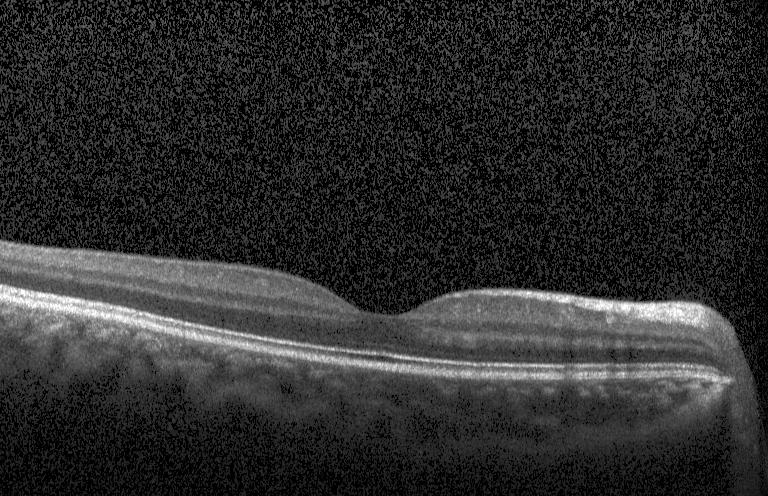

Acquired on a Heidelberg Spectralis · spectral-domain OCT · macular scan · retinal OCT cross-section. Impression: no evidence of choroidal neovascularization, diabetic macular edema, or drusen.